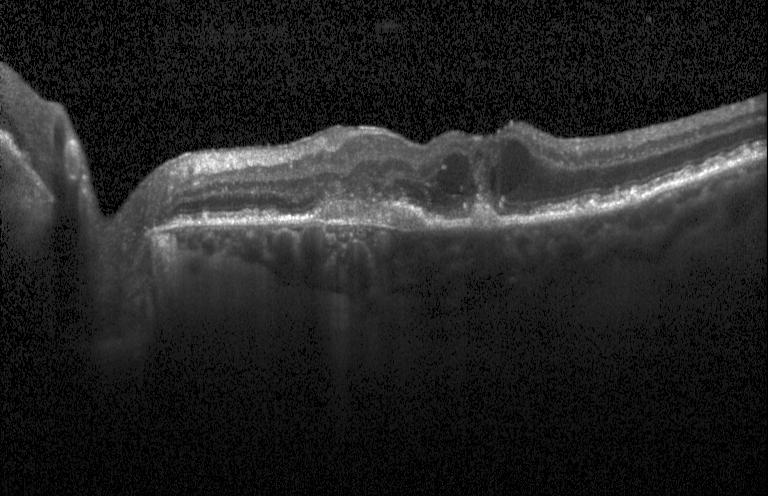 Retinal OCT B-scan, through the macula, Heidelberg Spectralis, SD-OCT — Dx: a choroidal neovascular membrane.